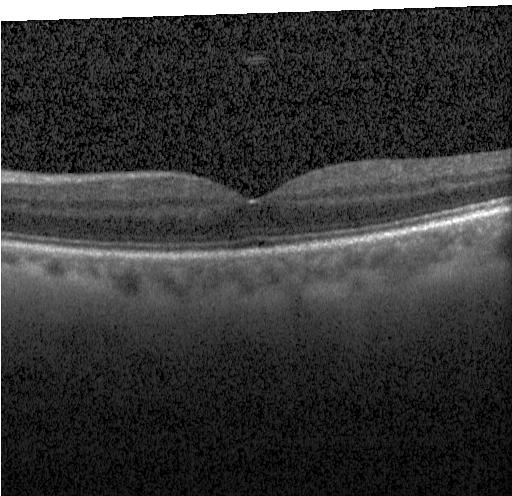

Retinal OCT B-scan · Heidelberg Spectralis OCT system — Dx: neither choroidal neovascularization, diabetic macular edema, nor drusen.